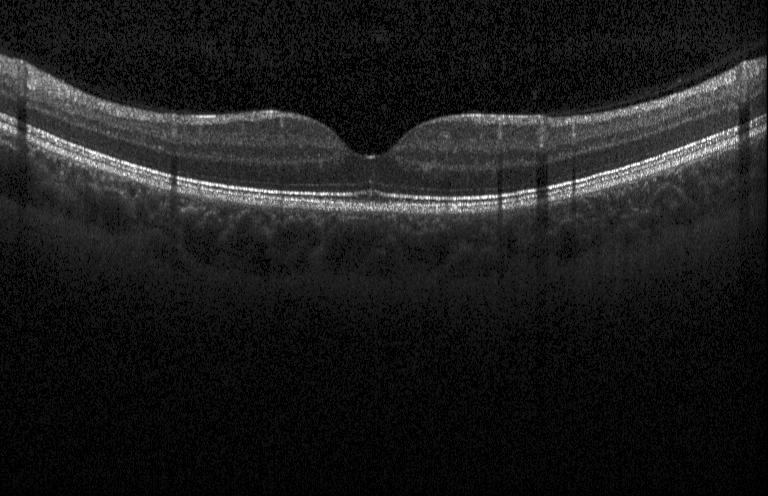
Fovea-centered, OCT line scan, spectral-domain optical coherence tomography, Heidelberg Spectralis
Assessment: neither CNV, DME, nor drusen.